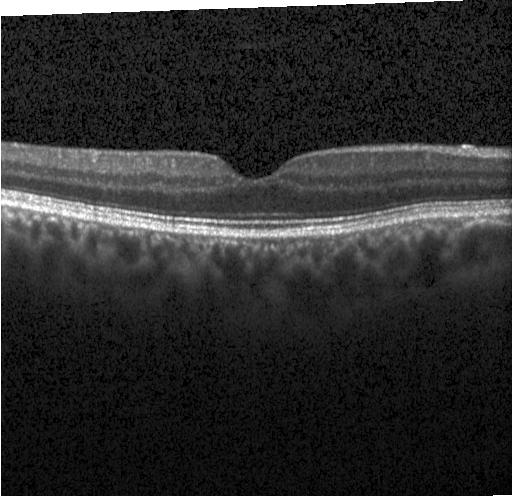
Assessment: no evidence of choroidal neovascularization, diabetic macular edema, or drusen.